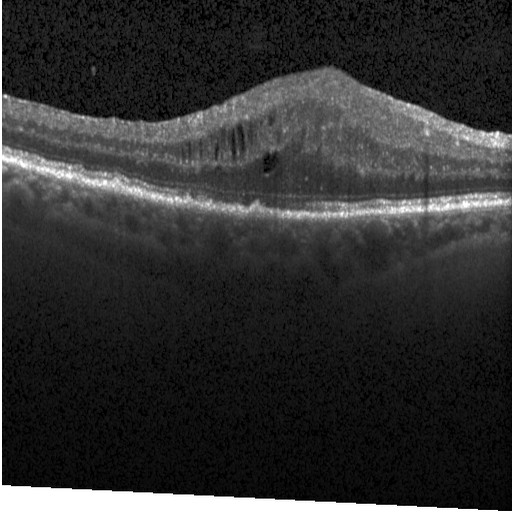
Macular OCT demonstrating DME.